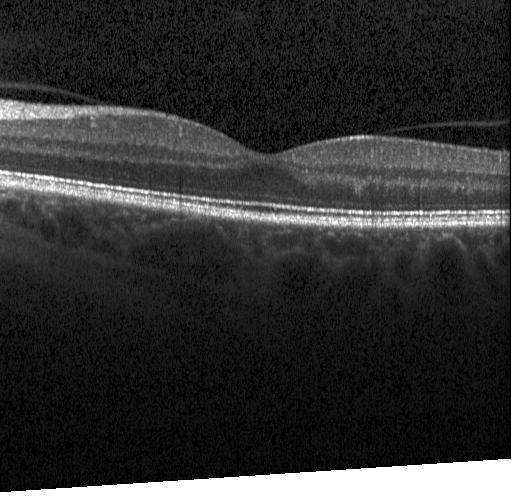

Neither choroidal neovascularization, diabetic macular edema, nor drusen.